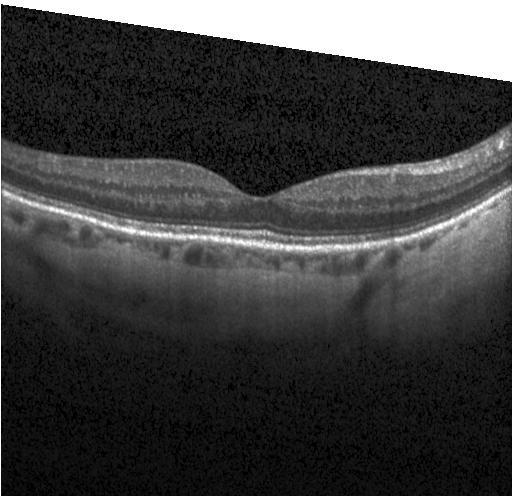

Optical coherence tomography B-scan, spectral-domain optical coherence tomography.
Impression: neither CNV, DME, nor drusen.